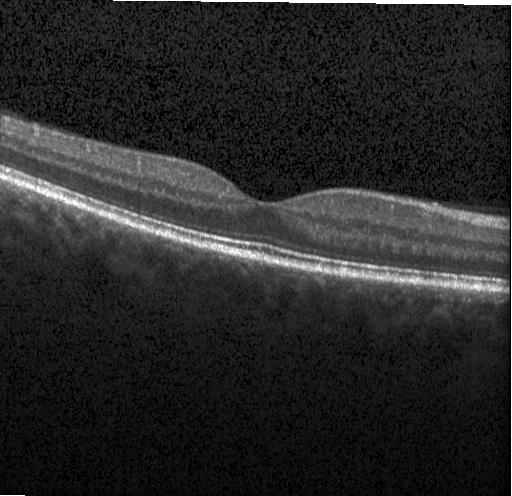
This B-scan demonstrates no choroidal neovascularization, no diabetic macular edema, and no drusen.